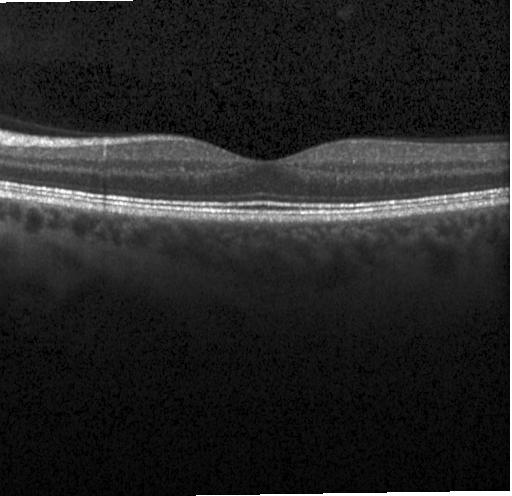

OCT B-scan. Neither choroidal neovascularization, diabetic macular edema, nor drusen.